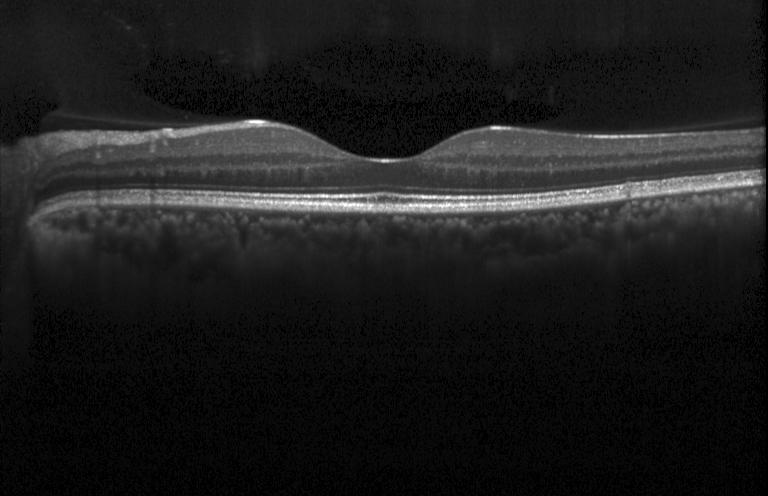

Diagnosis: no choroidal neovascularization, diabetic macular edema, or drusen.